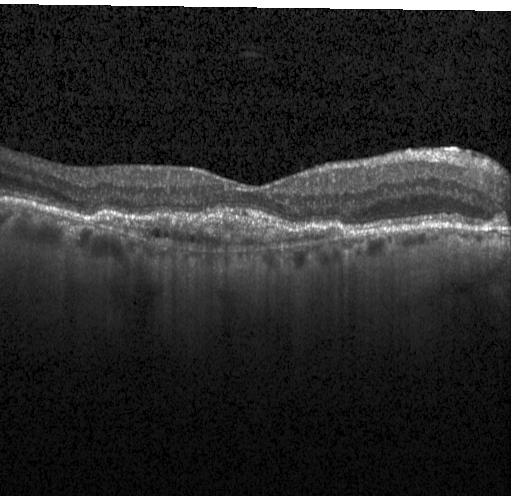 OCT line scan
Impression: a choroidal neovascular membrane.